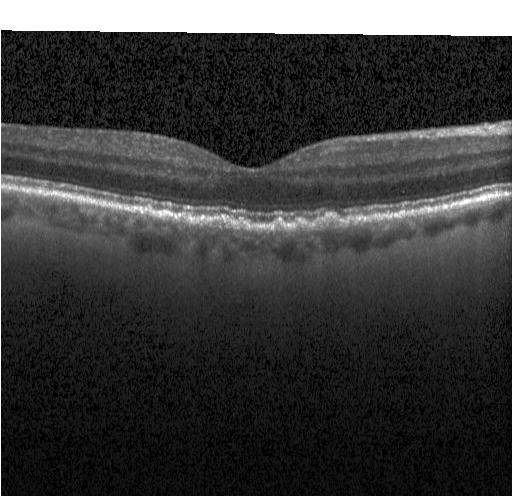 Retinal OCT cross-section. Macular OCT: sub-RPE drusenoid deposits.